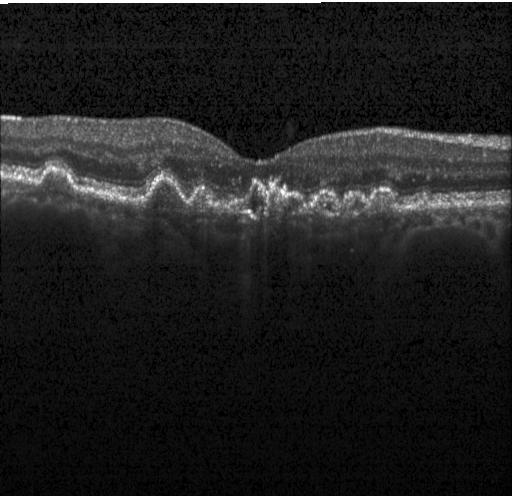
Optical coherence tomography B-scan — Diagnosis: CNV.